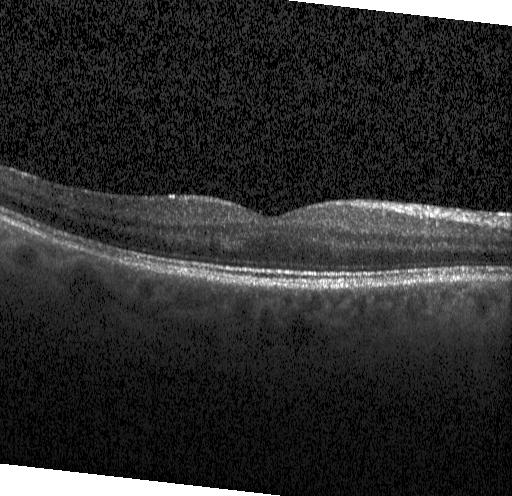
Optical coherence tomography scan — Diagnosis: no choroidal neovascularization, diabetic macular edema, or drusen.